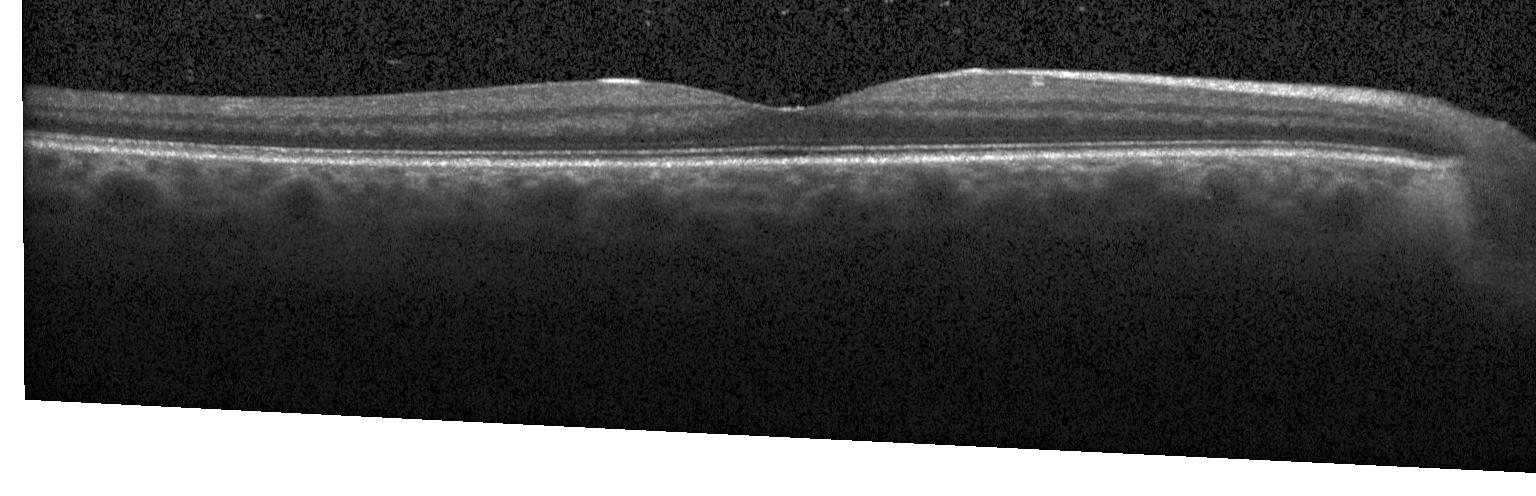
Optical coherence tomography B-scan, fovea-centered, Heidelberg Spectralis OCT system, spectral-domain OCT — Diagnosis: no evidence of choroidal neovascularization, diabetic macular edema, or drusen.